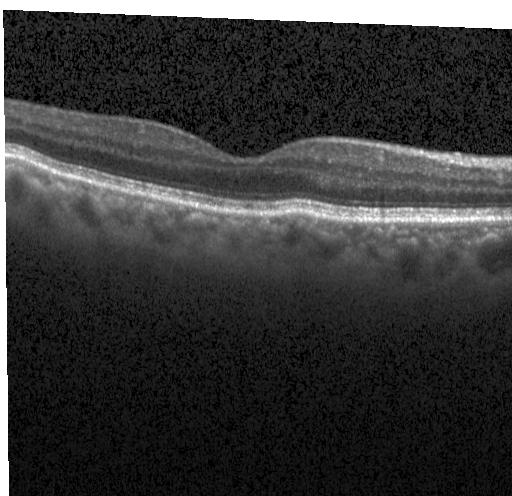
Spectral-domain optical coherence tomography. Optical coherence tomography scan. Through the macula
This B-scan demonstrates no choroidal neovascularization, no diabetic macular edema, and no drusen.